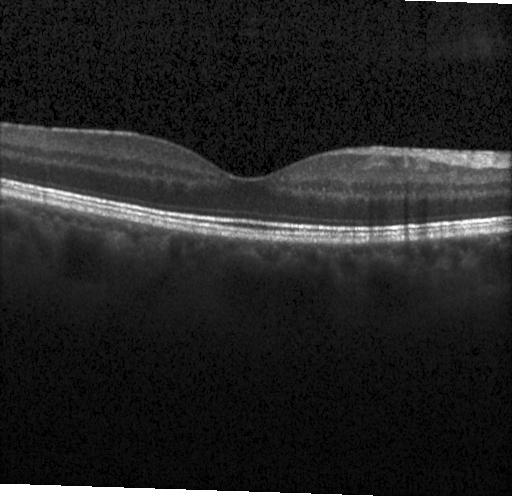
Optical coherence tomography B-scan. Instrument: Heidelberg Spectralis
Impression: no choroidal neovascularization, diabetic macular edema, or drusen.